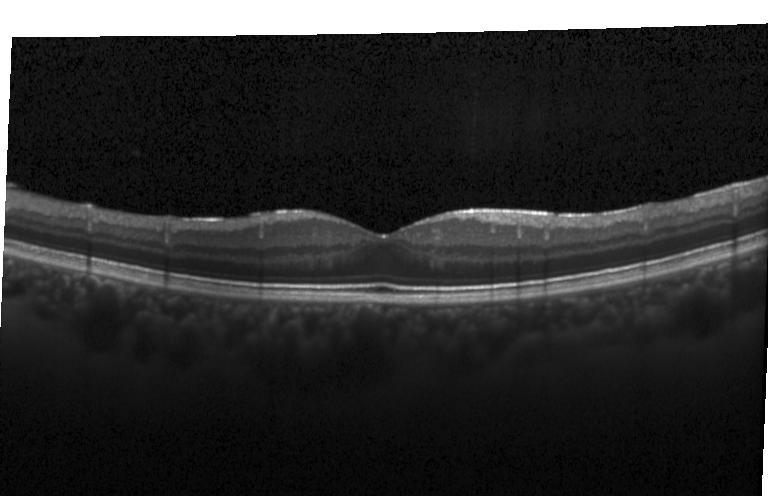
OCT B-scan; acquired on a Heidelberg Spectralis; centered on the fovea; spectral-domain OCT. No CNV, no DME, and no drusen.